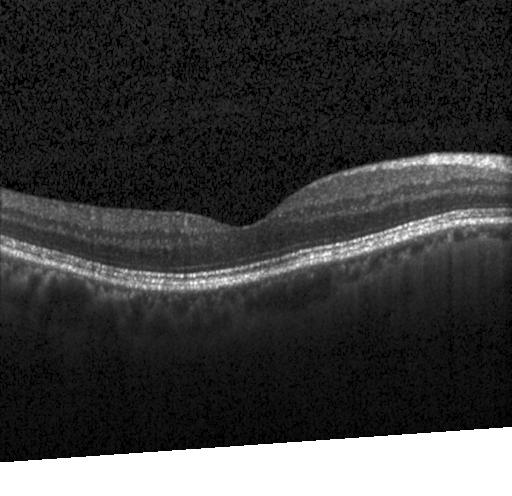

Neither choroidal neovascularization, diabetic macular edema, nor drusen.